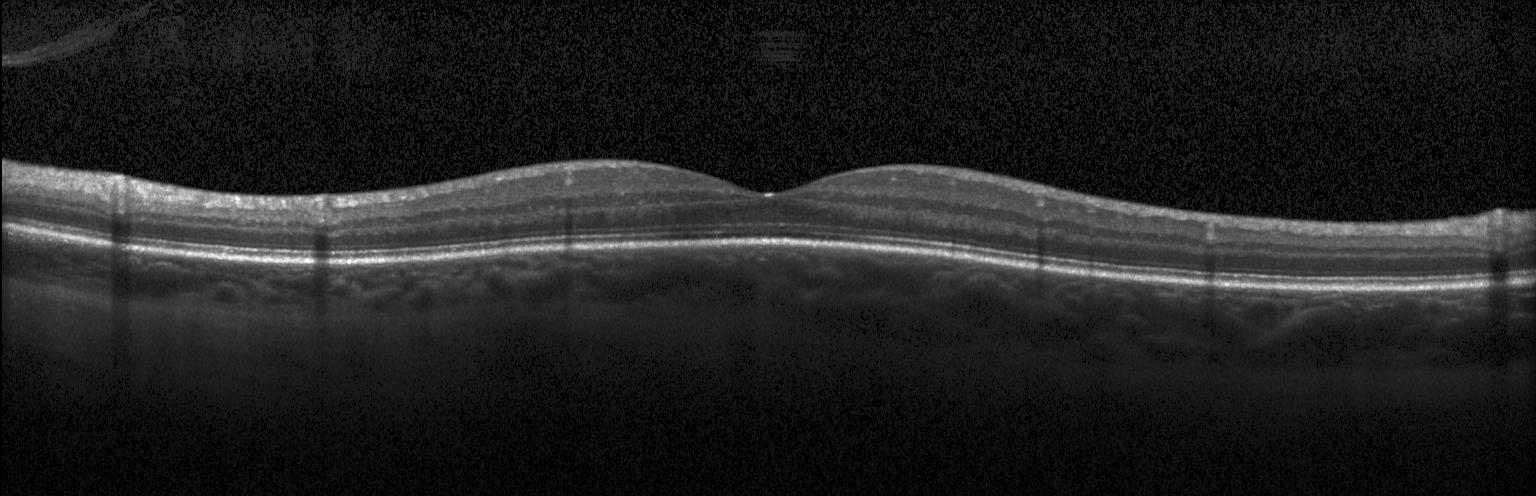
OCT B-scan showing no choroidal neovascularization, diabetic macular edema, or drusen.